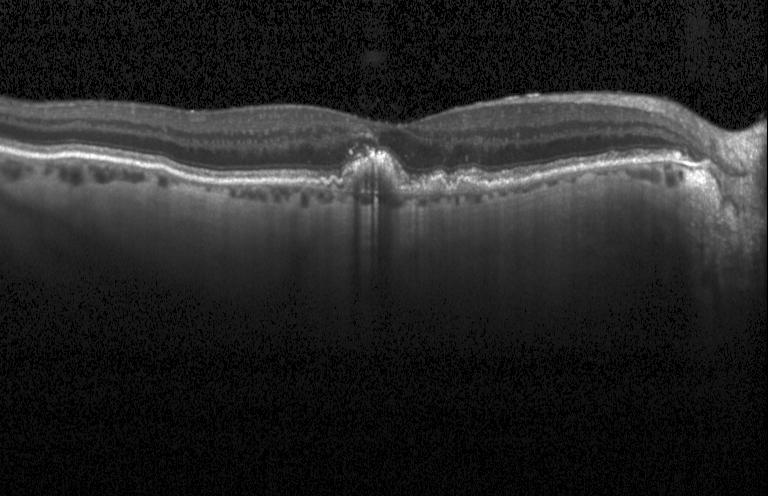

Horizontal scan through the fovea; retinal OCT cross-section. Macular OCT: multiple drusen.